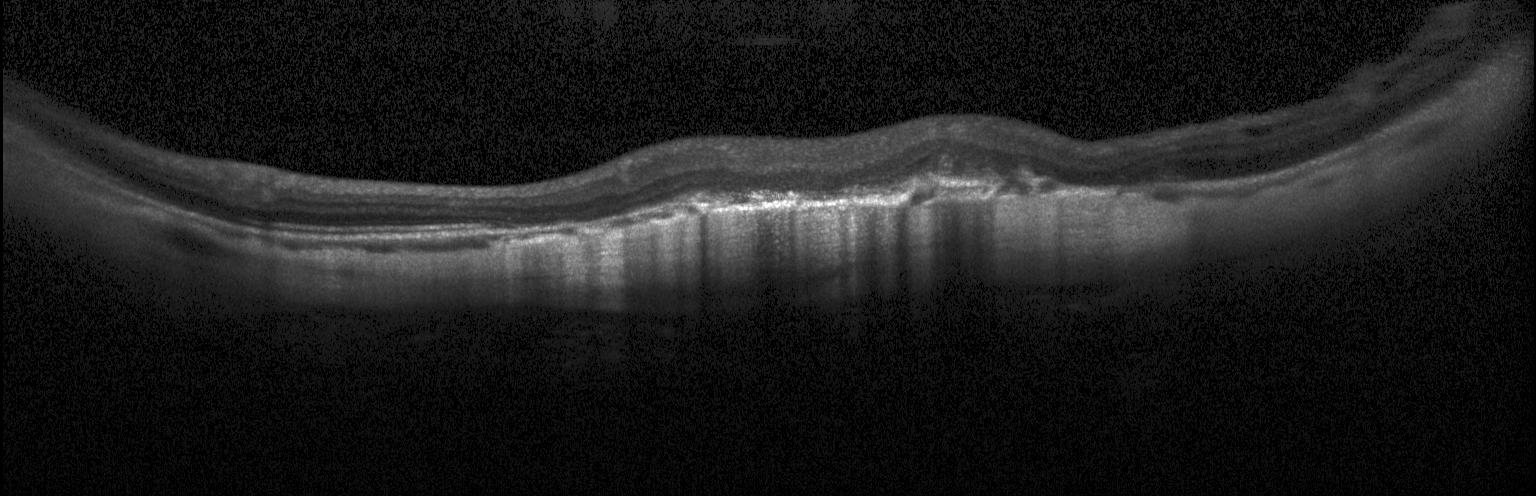
Heidelberg Spectralis; spectral-domain OCT; macular scan; optical coherence tomography B-scan — The scan shows CNV.